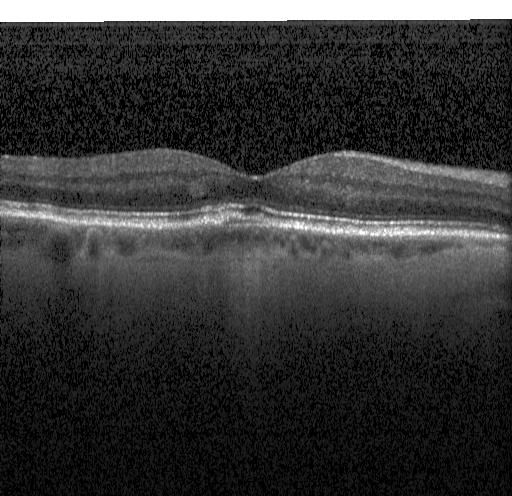
OCT line scan. Heidelberg Spectralis OCT system.
Finding: a choroidal neovascular membrane.